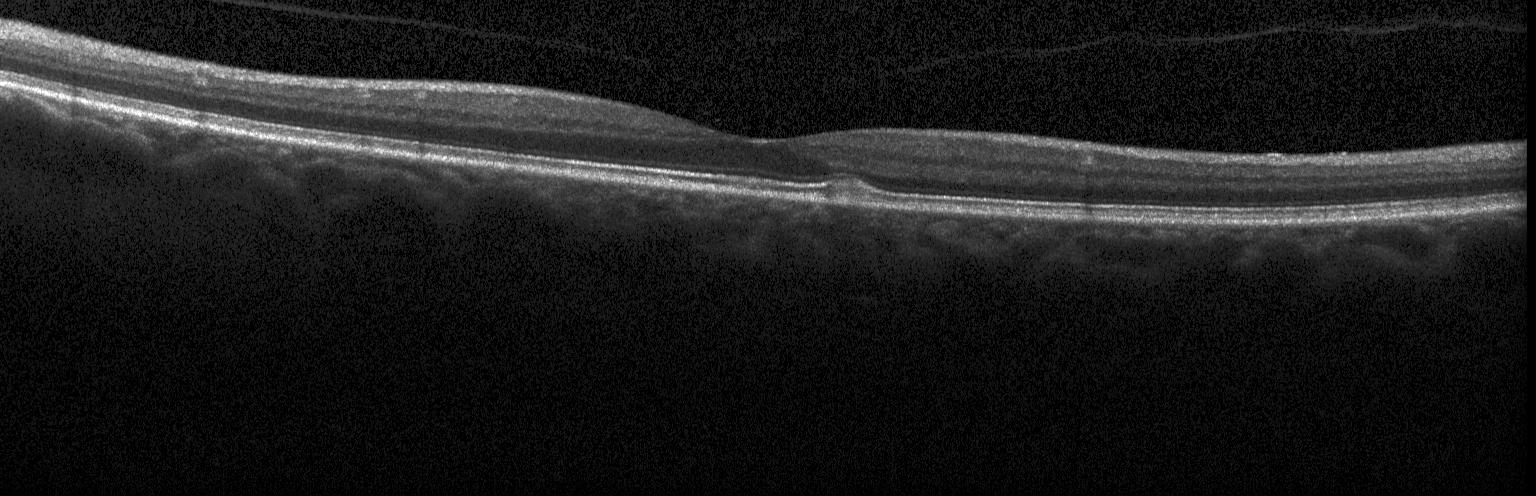 OCT B-scan showing neither CNV, DME, nor drusen.